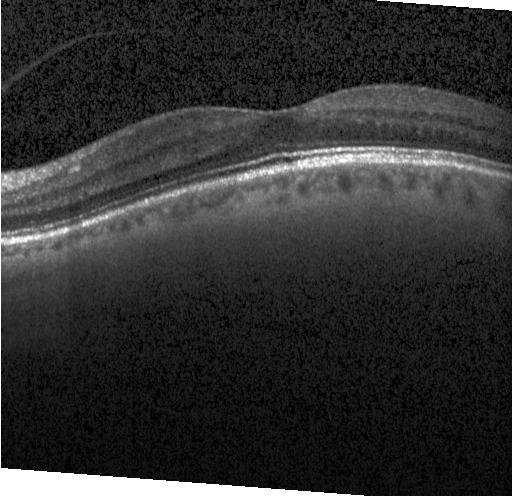 Through the macula; retinal OCT cross-section; Heidelberg Spectralis; spectral-domain OCT — Finding: no evidence of CNV, DME, or drusen.